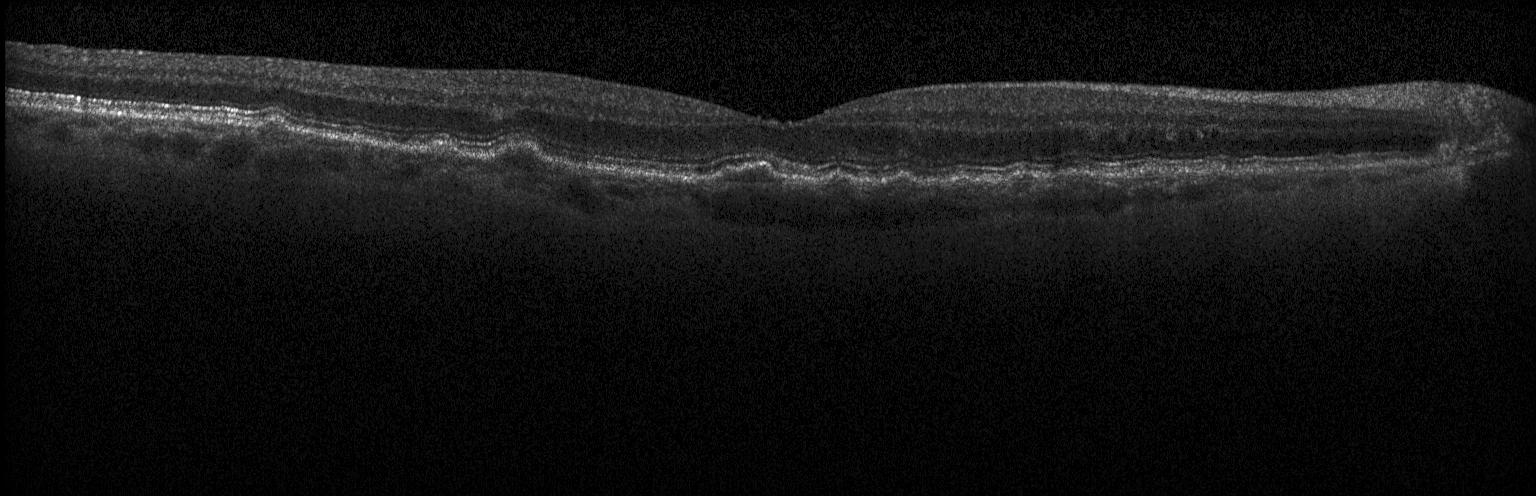
Multiple drusen.